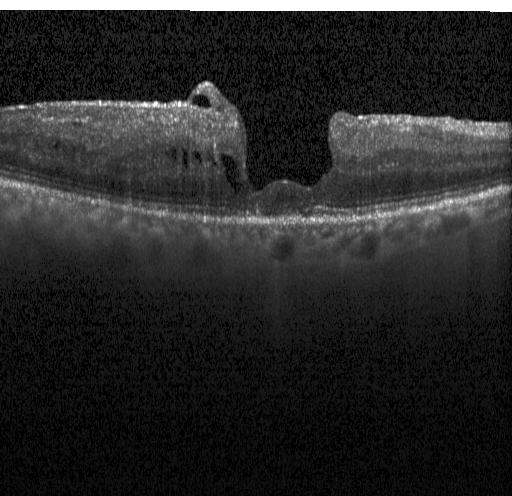

OCT line scan — Finding: DME.